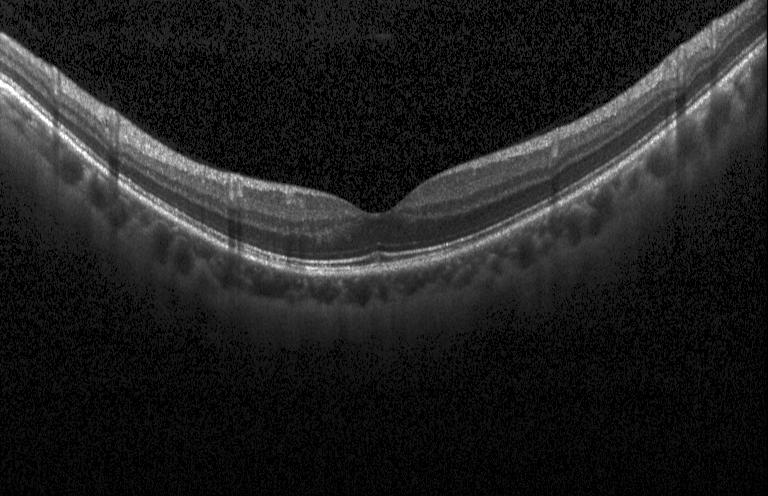
Impression: no choroidal neovascularization, no diabetic macular edema, and no drusen.